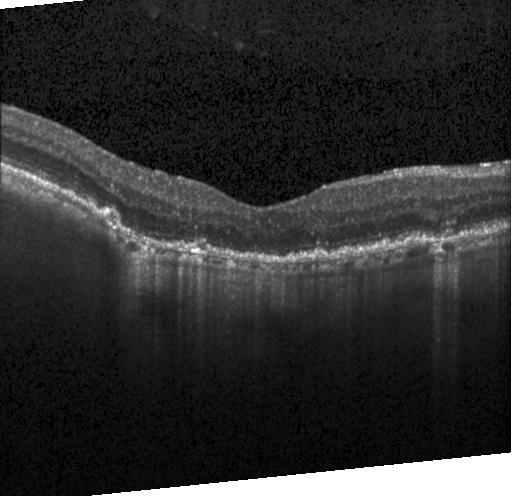

Retinal OCT cross-section showing a choroidal neovascular membrane.